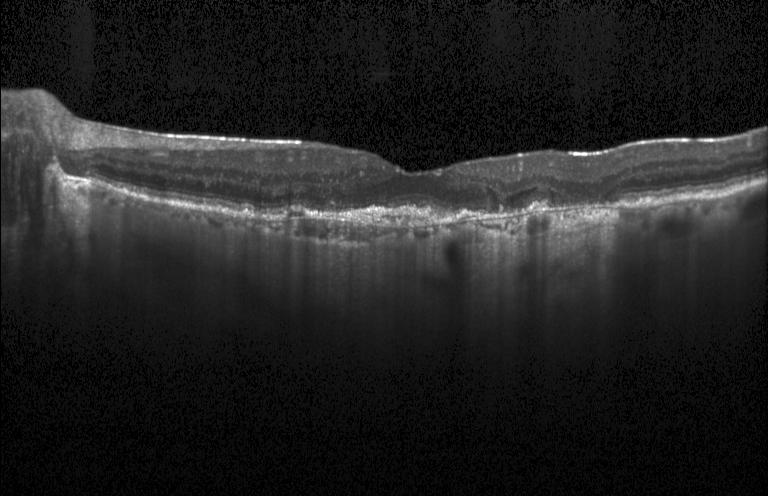
Heidelberg Spectralis; retinal OCT B-scan — Macular OCT: a choroidal neovascular membrane.